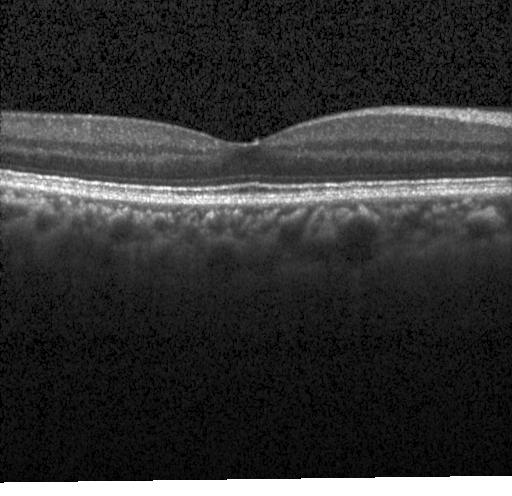

Optical coherence tomography scan; acquired on a Heidelberg Spectralis
No evidence of choroidal neovascularization, diabetic macular edema, or drusen.